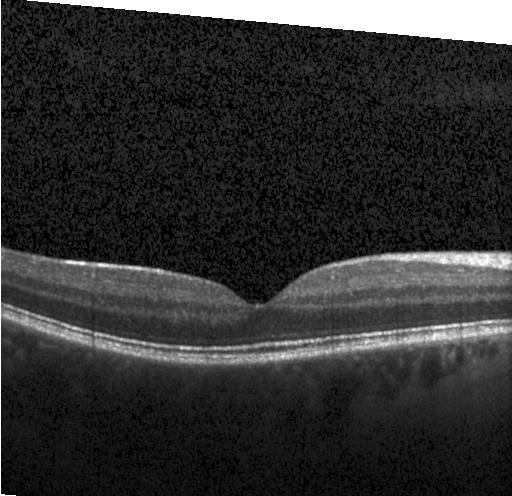
OCT B-scan. Macular OCT: neither choroidal neovascularization, diabetic macular edema, nor drusen.